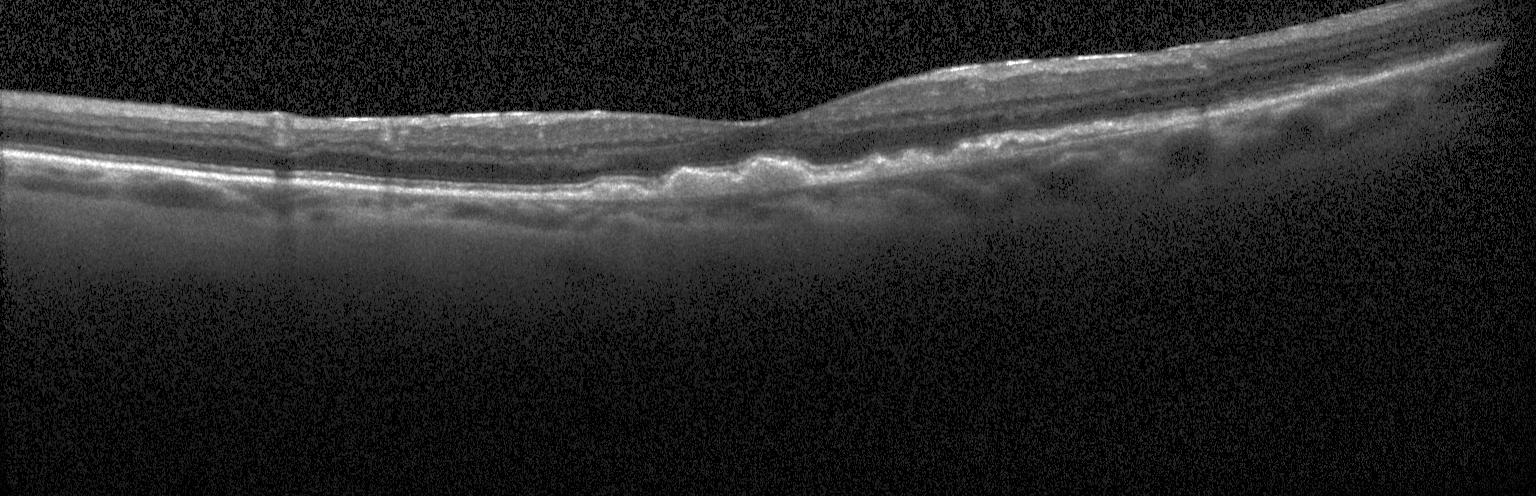
Finding: sub-RPE drusenoid deposits.